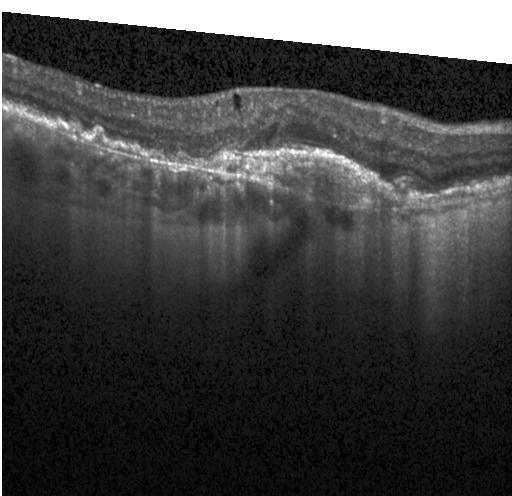 Spectral-domain OCT, Heidelberg Spectralis, OCT B-scan
Impression: a choroidal neovascular membrane.